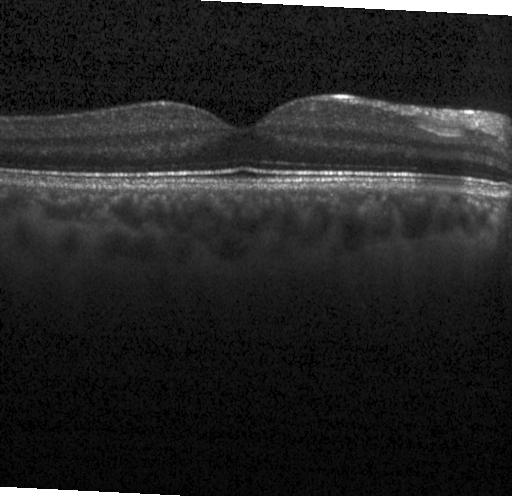

OCT B-scan.
Macular OCT: no evidence of choroidal neovascularization, diabetic macular edema, or drusen.